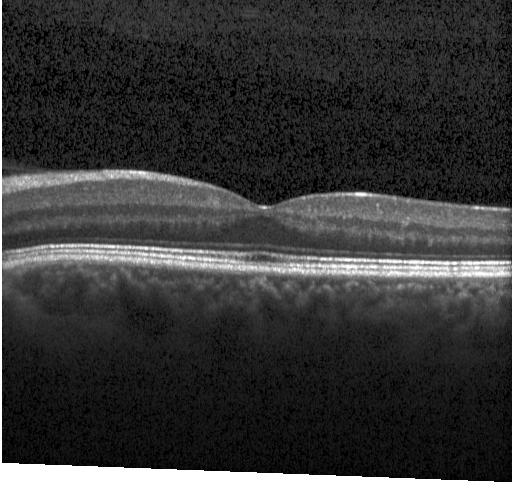
Optical coherence tomography scan.
Diagnosis: no evidence of choroidal neovascularization, diabetic macular edema, or drusen.